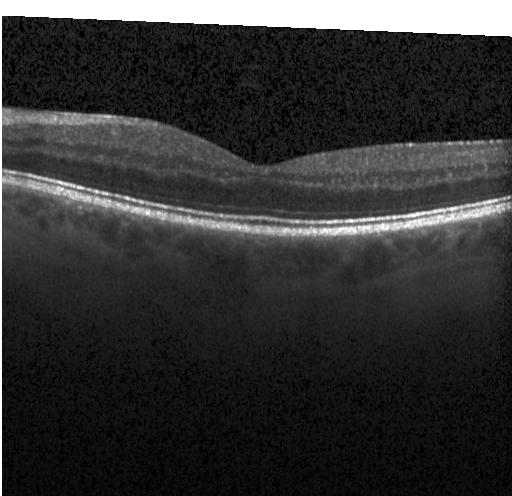
Optical coherence tomography scan · spectral-domain optical coherence tomography. Macular OCT: neither CNV, DME, nor drusen.